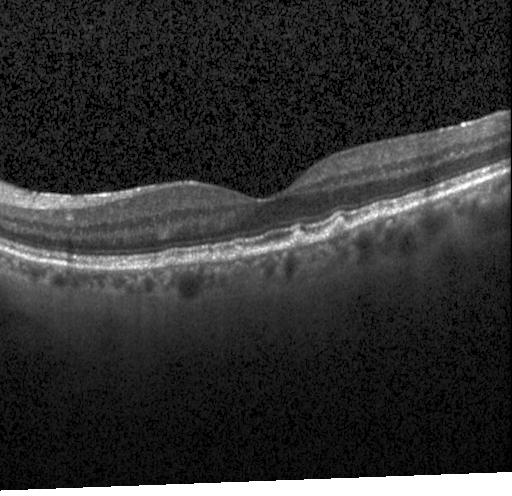 Spectral-domain OCT · fovea-centered · retinal OCT cross-section · acquired on a Heidelberg Spectralis — The scan shows drusen.